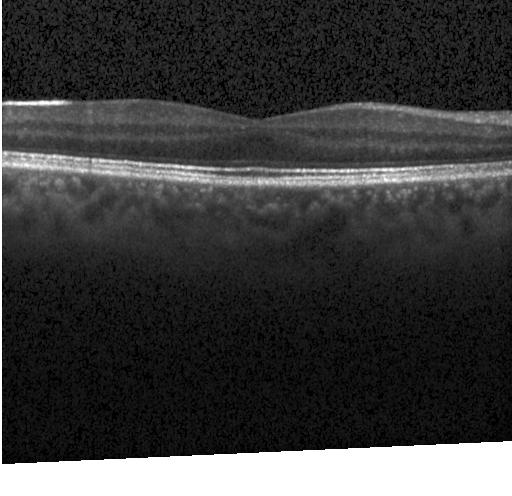
OCT B-scan showing no evidence of choroidal neovascularization, diabetic macular edema, or drusen.